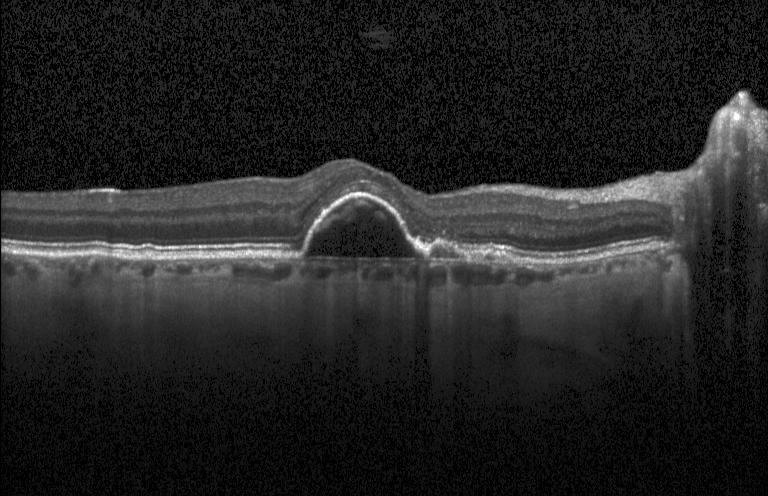
Optical coherence tomography B-scan; Heidelberg Spectralis; spectral-domain optical coherence tomography.
Finding: CNV.